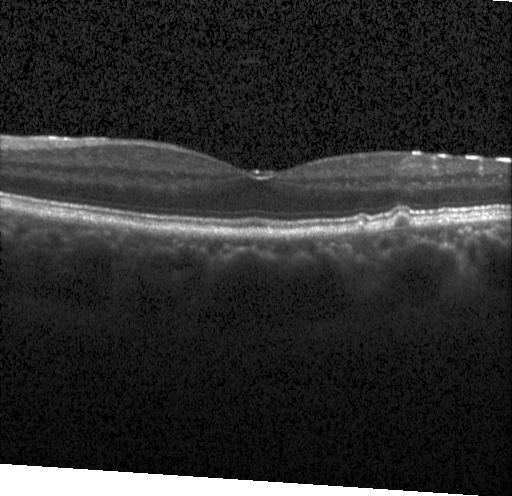
The scan shows multiple drusen.